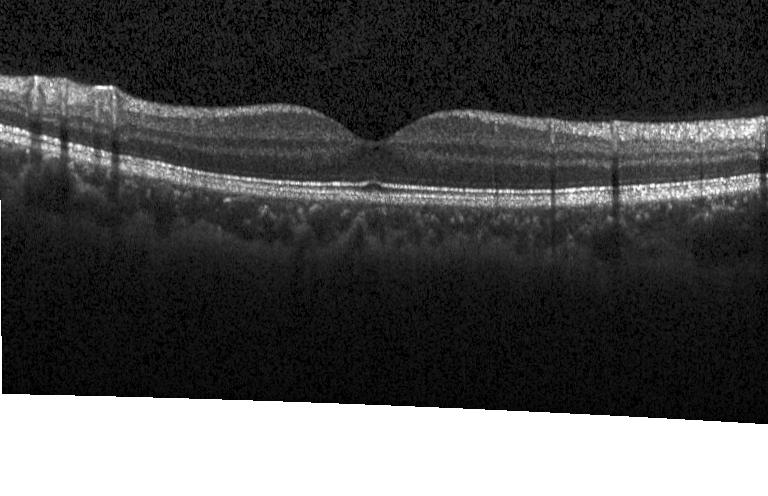
Finding: no evidence of choroidal neovascularization, diabetic macular edema, or drusen.